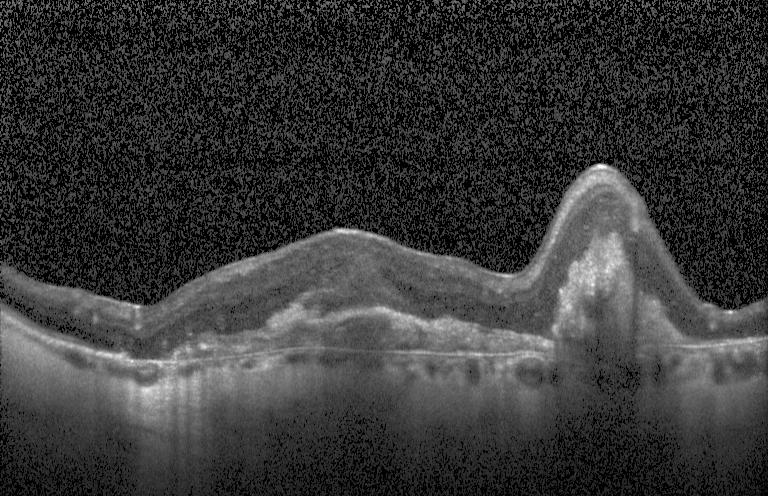 Retinal OCT B-scan · through the macula · instrument: Heidelberg Spectralis · SD-OCT
Finding: a choroidal neovascular membrane.